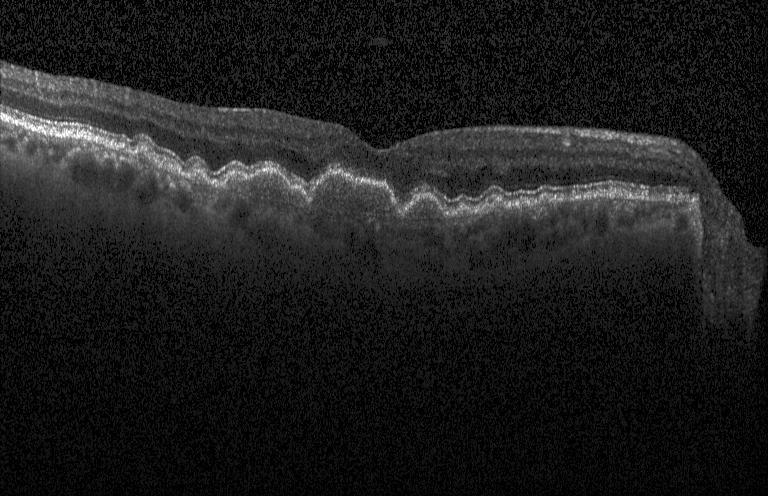

Diagnosis: drusen.